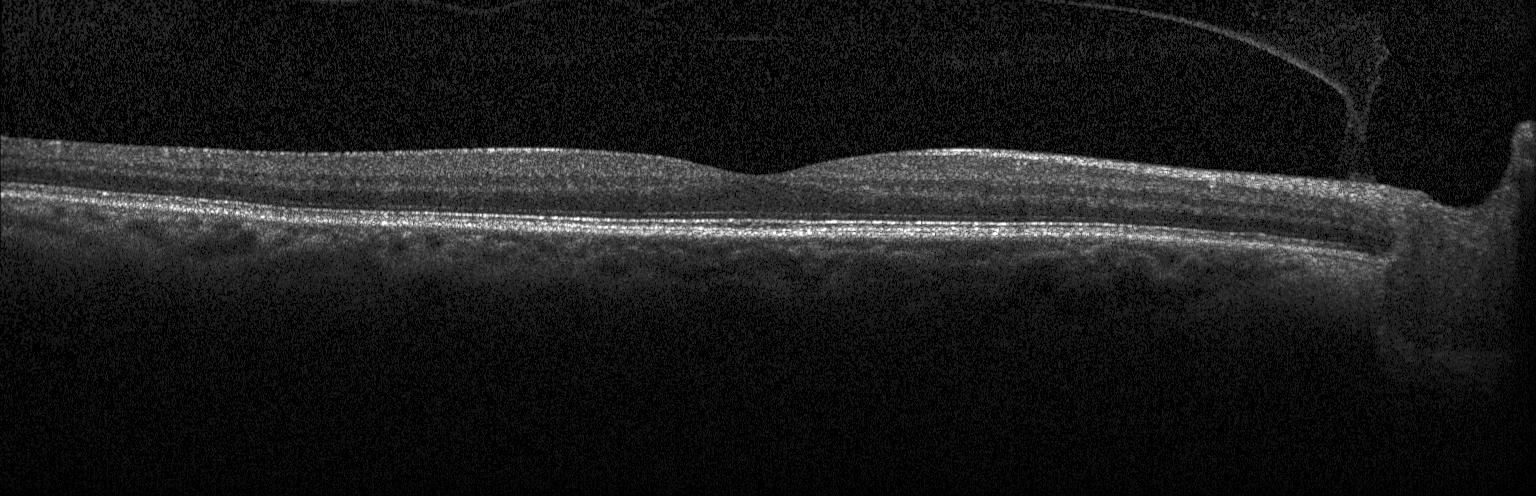

OCT B-scan — Finding: no evidence of choroidal neovascularization, diabetic macular edema, or drusen.